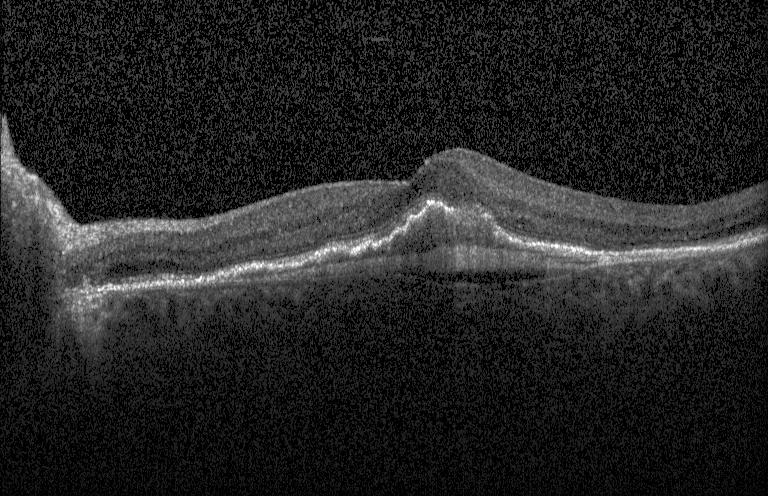
Spectral-domain OCT B-scan: a choroidal neovascular membrane.